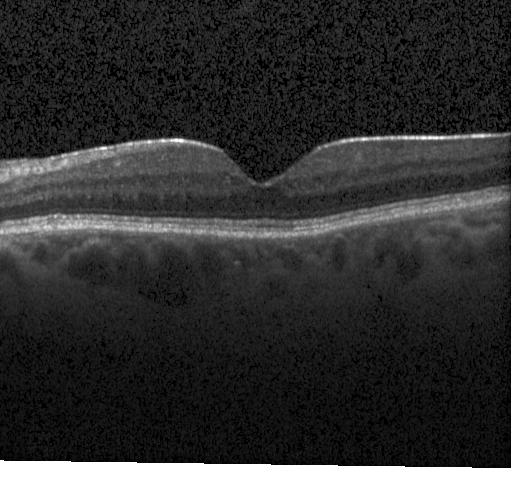 Macular OCT: no evidence of choroidal neovascularization, diabetic macular edema, or drusen.